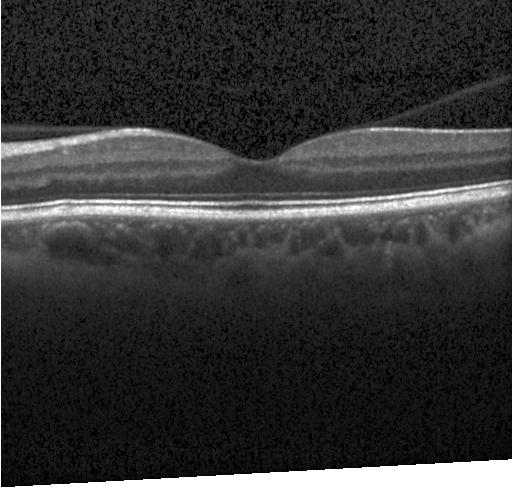
SD-OCT. OCT line scan. Centered on the fovea. Finding: neither CNV, DME, nor drusen.